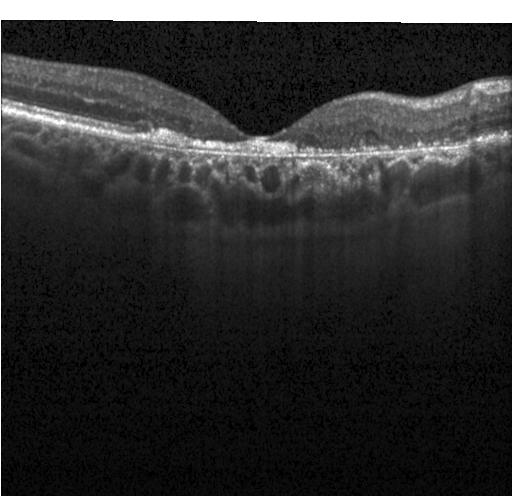

OCT line scan; macular scan; spectral-domain OCT.
Assessment: a choroidal neovascular membrane.